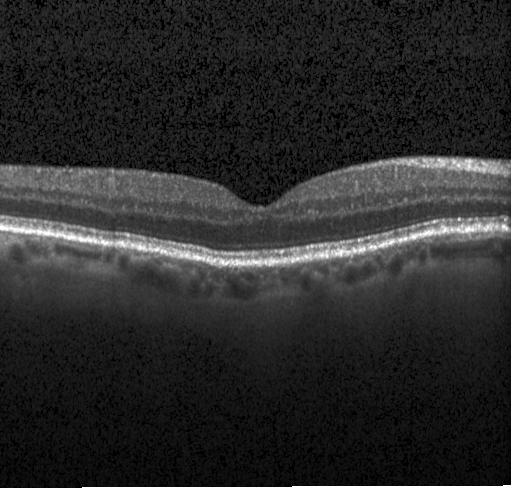 Spectral-domain OCT. OCT B-scan. Fovea-centered. Diagnosis: no evidence of choroidal neovascularization, diabetic macular edema, or drusen.